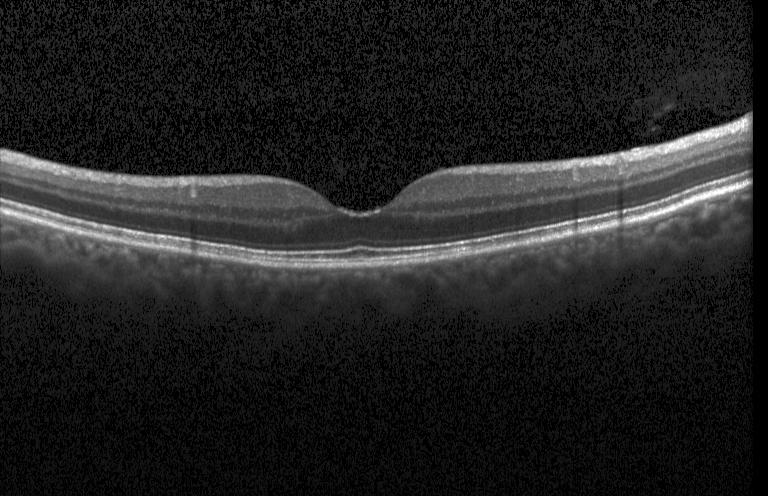 Heidelberg Spectralis OCT system · optical coherence tomography B-scan — No CNV, no DME, and no drusen.